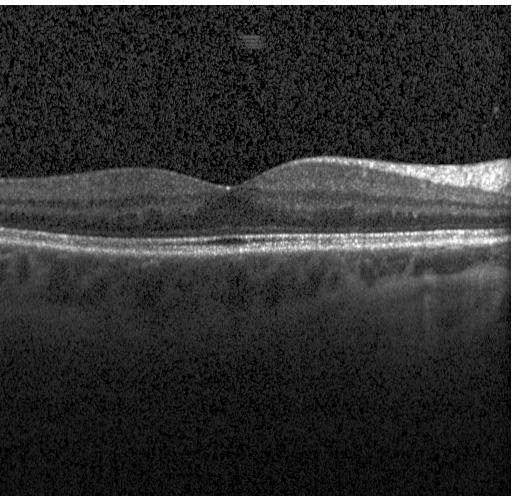
Impression: neither CNV, DME, nor drusen.